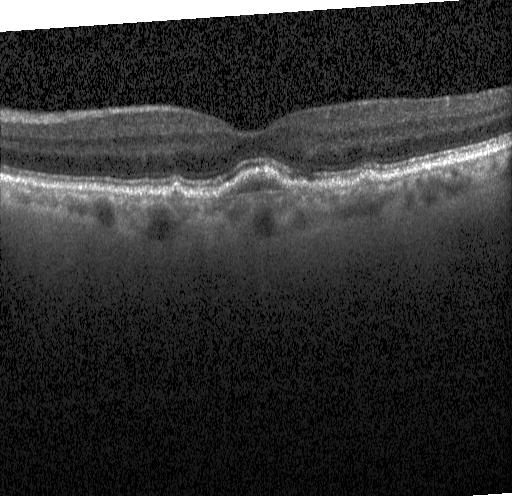

The scan shows a choroidal neovascular membrane.